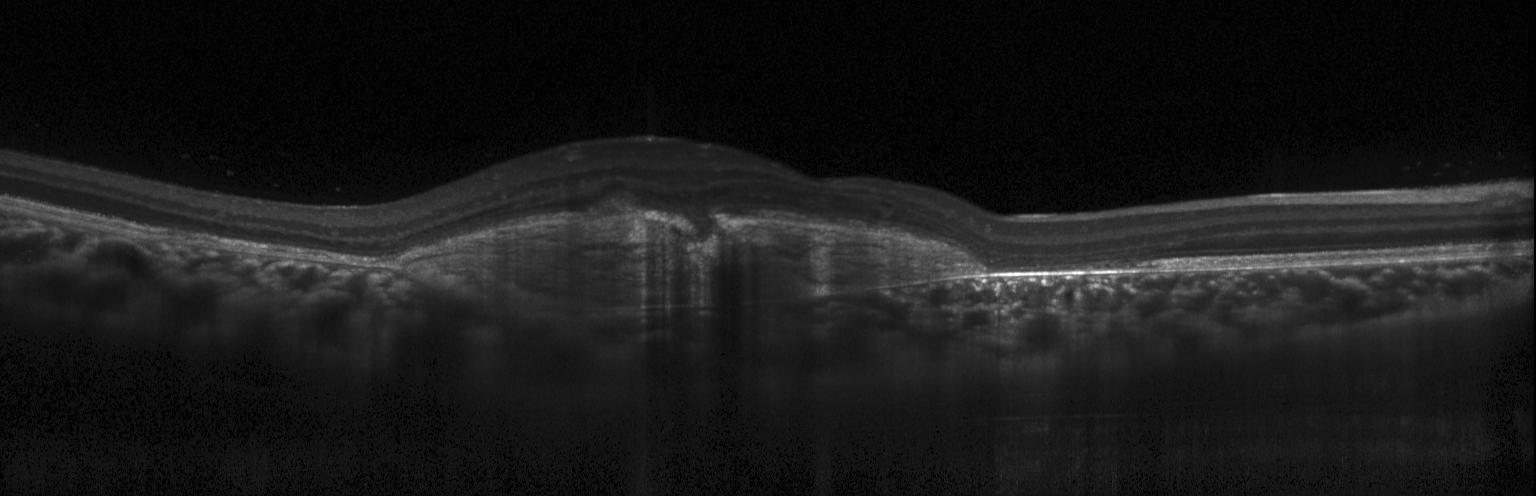

Optical coherence tomography B-scan — Macular OCT: a choroidal neovascular membrane.